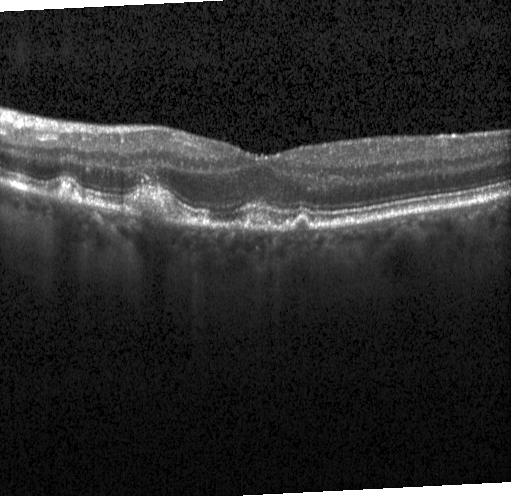 Retinal OCT B-scan. The scan shows choroidal neovascularization.